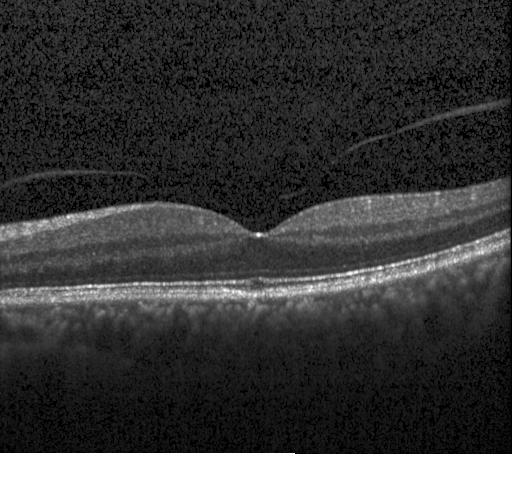 Impression: neither choroidal neovascularization, diabetic macular edema, nor drusen.